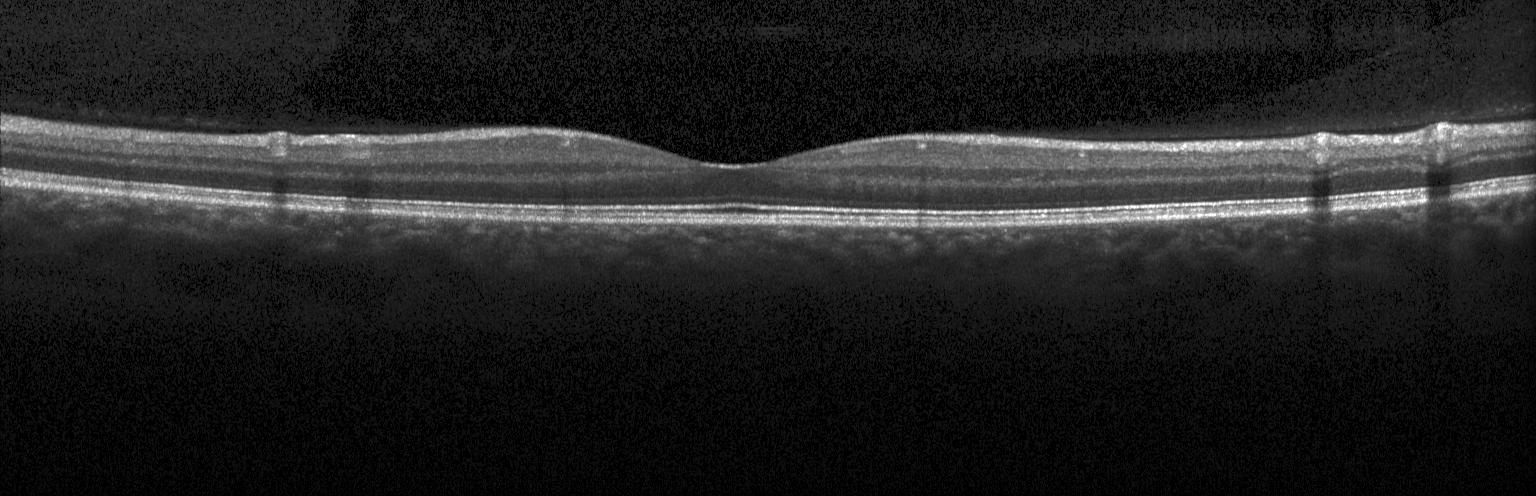 Acquired on a Heidelberg Spectralis. OCT B-scan. Spectral-domain optical coherence tomography. Horizontal scan through the fovea — Dx: no CNV, no DME, and no drusen.